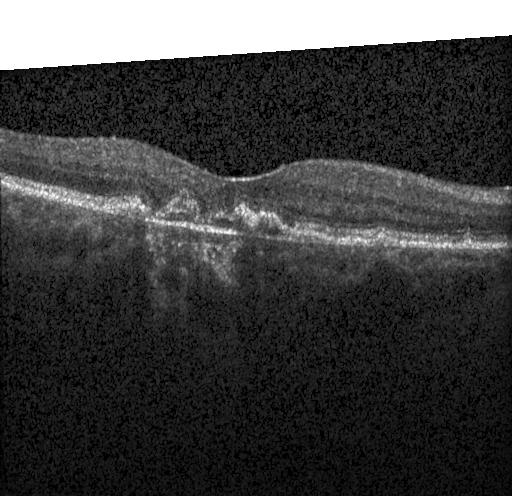
Diagnosis: CNV.